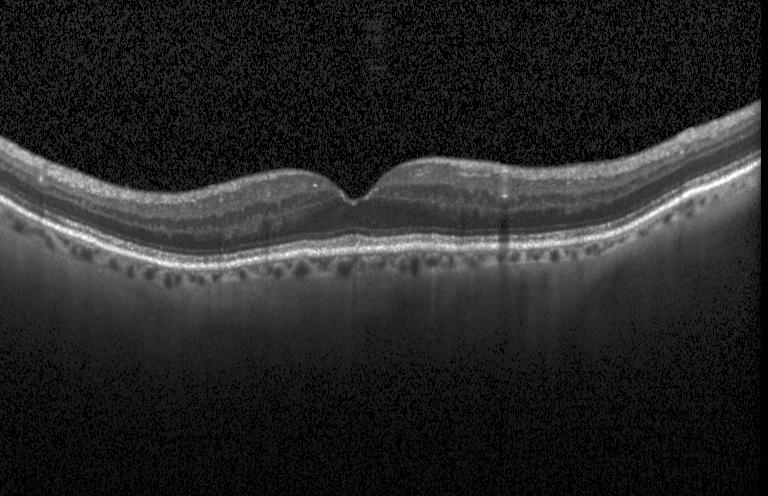 Spectral-domain OCT, optical coherence tomography B-scan — Finding: neither CNV, DME, nor drusen.